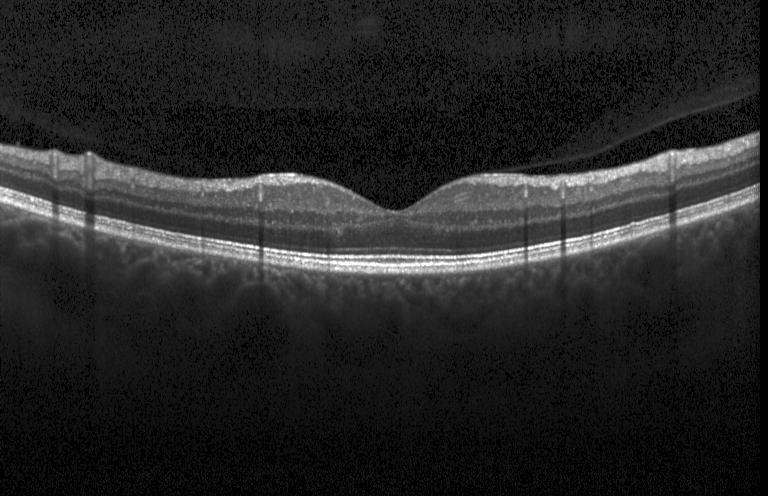
Optical coherence tomography B-scan.
Dx: no CNV, DME, or drusen.